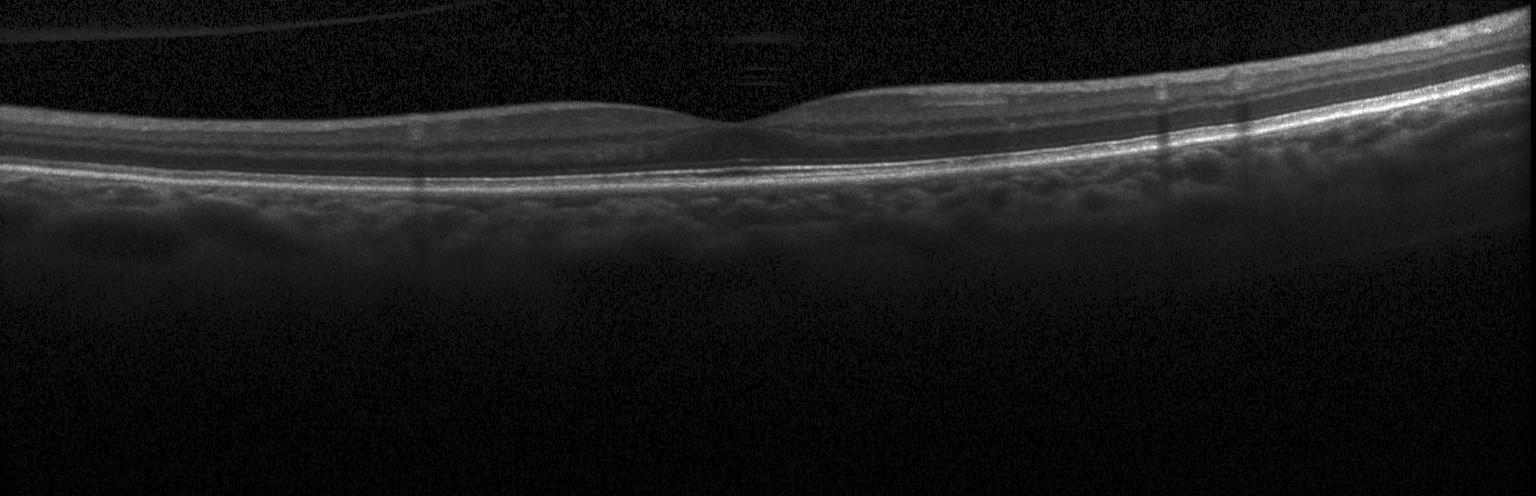

Macular OCT: no choroidal neovascularization, no diabetic macular edema, and no drusen.